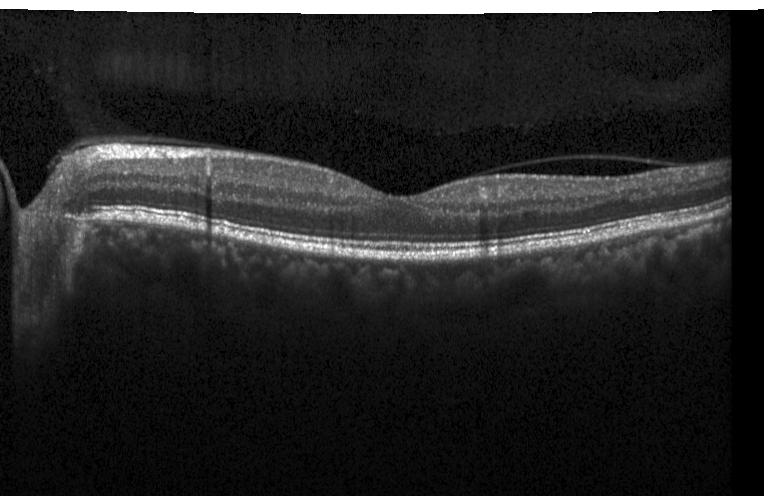 Assessment: no CNV, DME, or drusen.